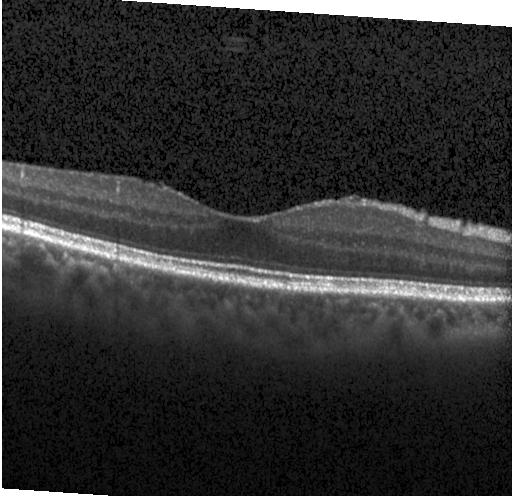 OCT B-scan. Fovea-centered. SD-OCT. Acquired on a Heidelberg Spectralis
Assessment: no choroidal neovascularization, diabetic macular edema, or drusen.